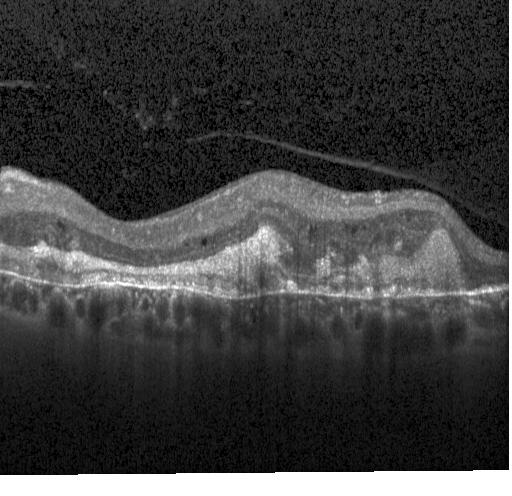
Optical coherence tomography B-scan; instrument: Heidelberg Spectralis — This B-scan demonstrates a choroidal neovascular membrane.